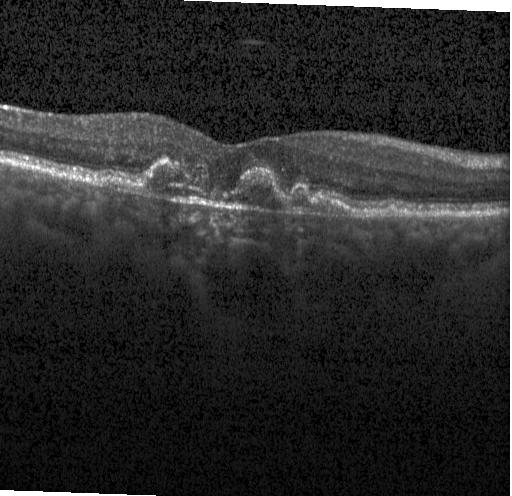 Retinal OCT B-scan · Heidelberg Spectralis · macular scan
The scan shows choroidal neovascularization.